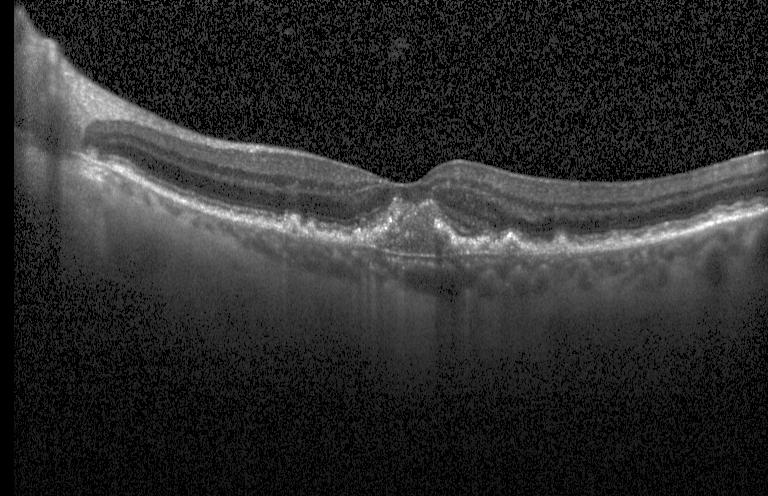

Retinal OCT B-scan; macular scan; SD-OCT; instrument: Heidelberg Spectralis.
The scan shows choroidal neovascularization.